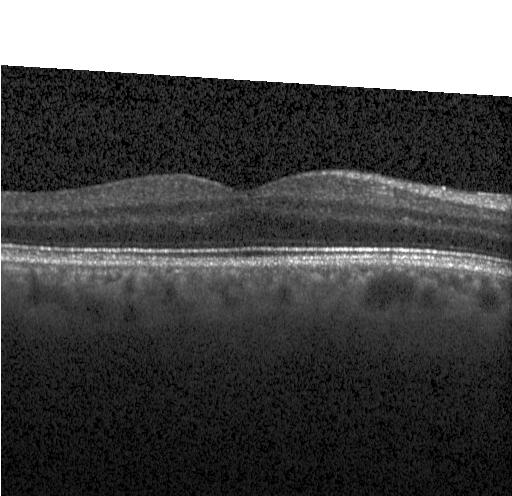

Macular scan, Heidelberg Spectralis OCT system, optical coherence tomography B-scan.
Finding: no choroidal neovascularization, no diabetic macular edema, and no drusen.